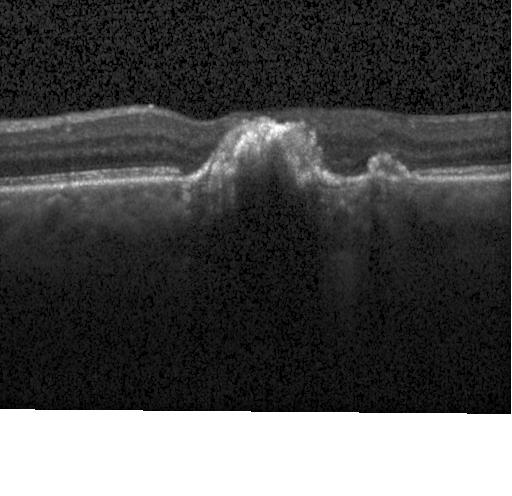

Finding: a choroidal neovascular membrane.